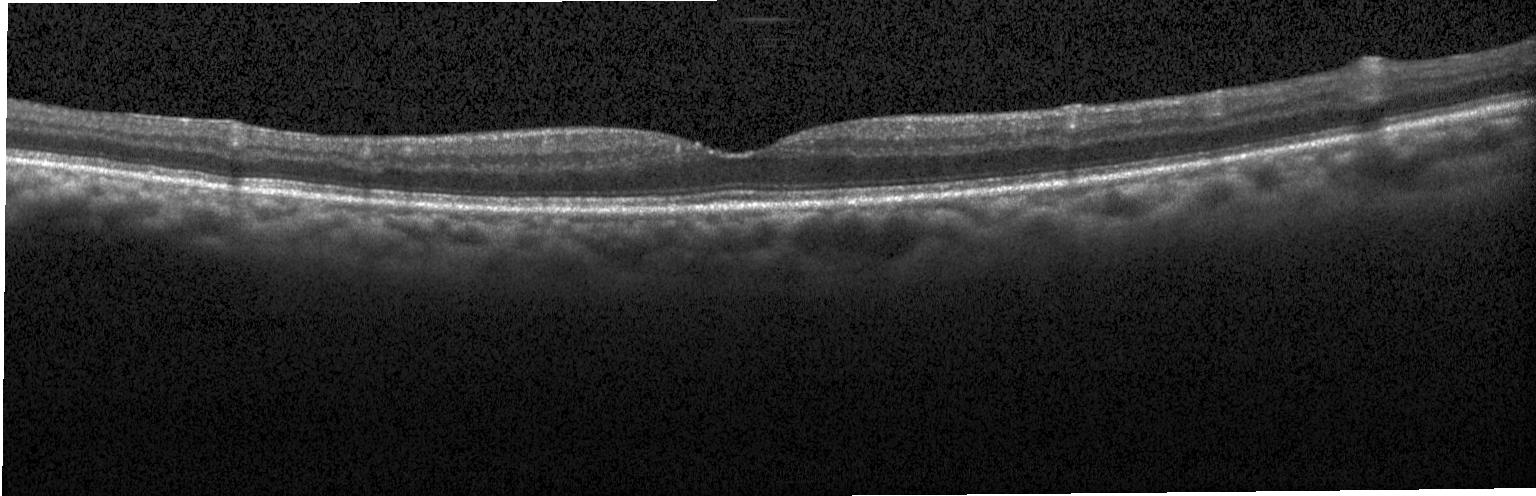 OCT B-scan.
OCT finding: no evidence of choroidal neovascularization, diabetic macular edema, or drusen.